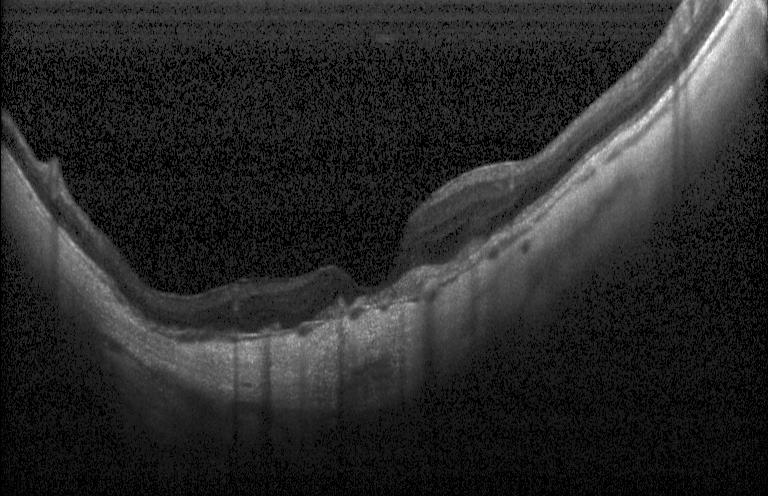
OCT finding: a choroidal neovascular membrane.